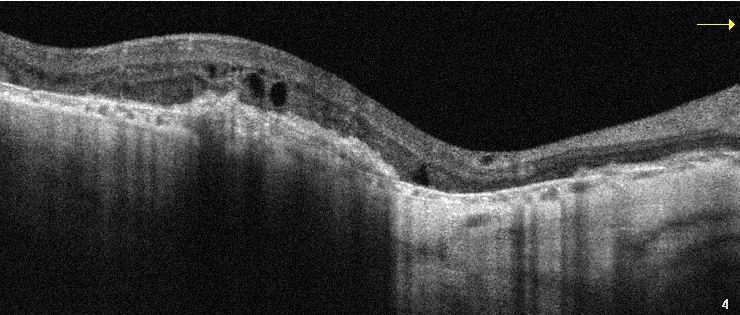
Retinal OCT B-scan
This B-scan demonstrates AMD.